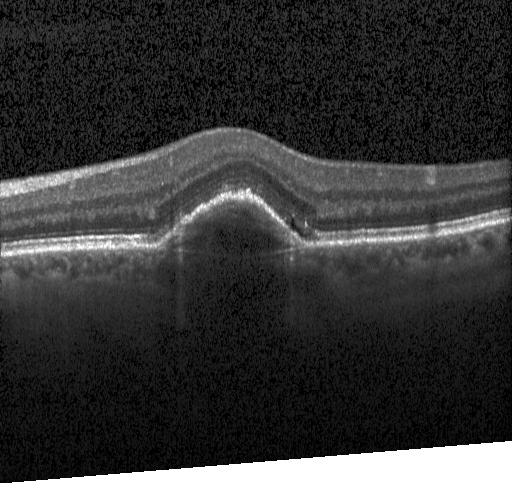 Spectral-domain OCT, acquired on a Heidelberg Spectralis, retinal OCT cross-section, through the macula. Finding: a choroidal neovascular membrane.